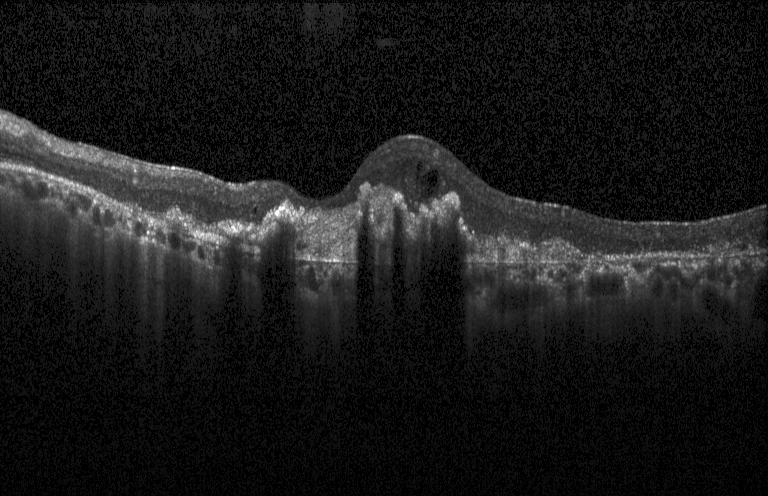

Dx: choroidal neovascularization.